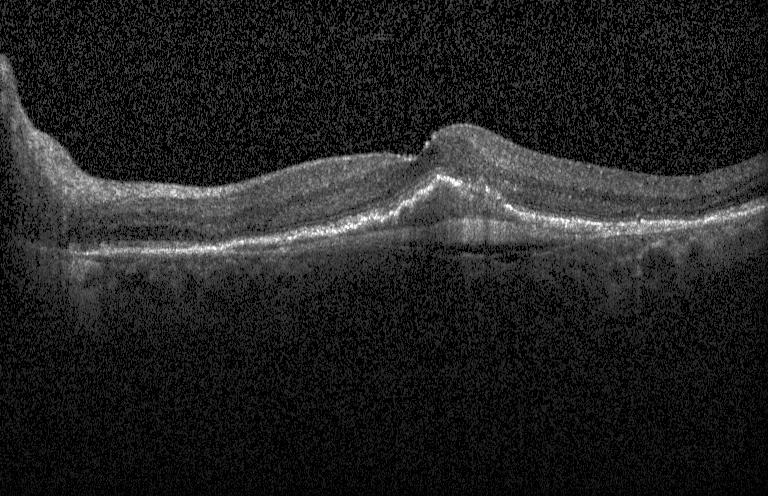
Impression: CNV.